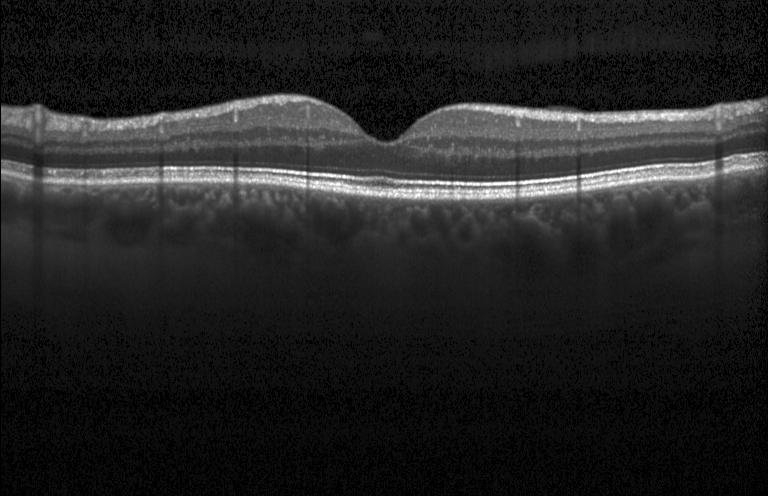

Fovea-centered · instrument: Heidelberg Spectralis · OCT B-scan — Diagnosis: no choroidal neovascularization, no diabetic macular edema, and no drusen.